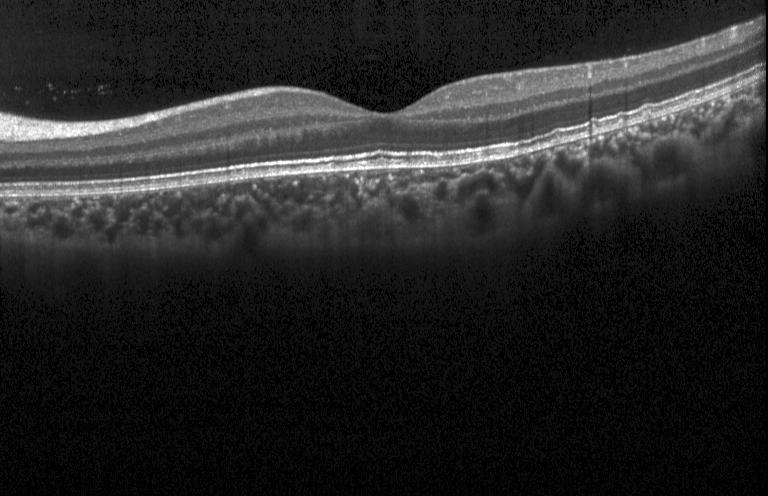 Heidelberg Spectralis, retinal OCT cross-section
Neither choroidal neovascularization, diabetic macular edema, nor drusen.